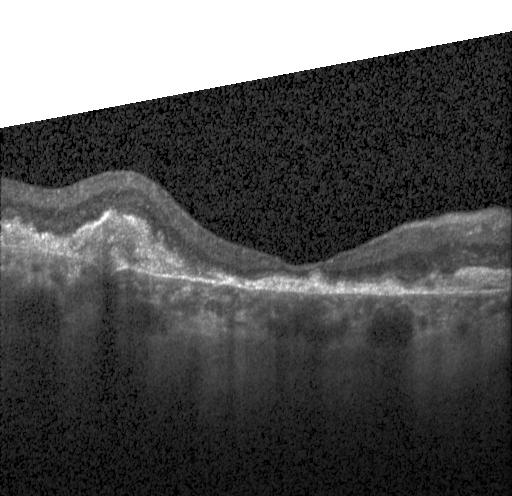

Spectral-domain OCT B-scan: choroidal neovascularization.